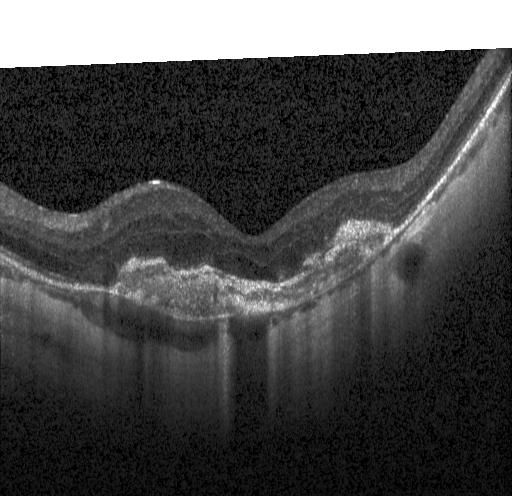
This B-scan demonstrates a choroidal neovascular membrane.